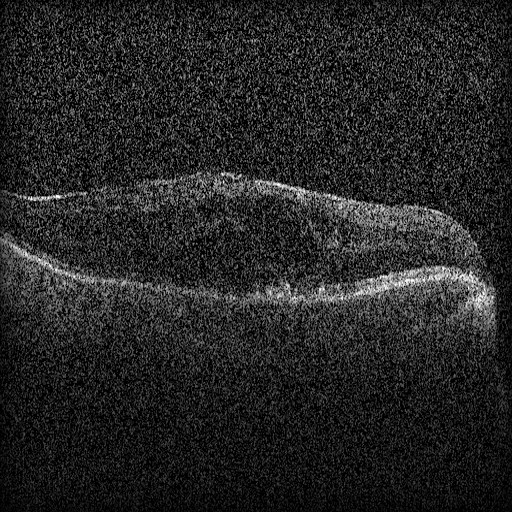

Diabetic macular edema.